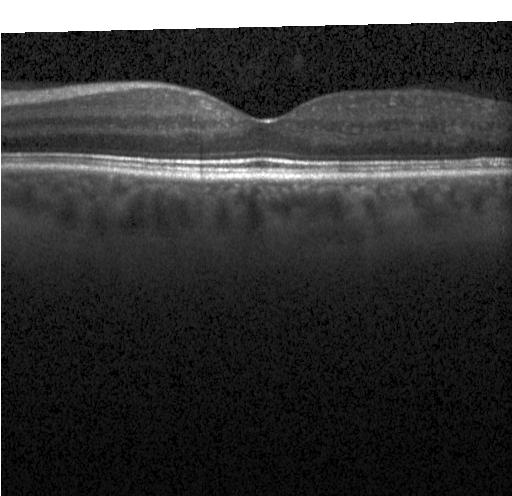 Diagnosis: neither choroidal neovascularization, diabetic macular edema, nor drusen.